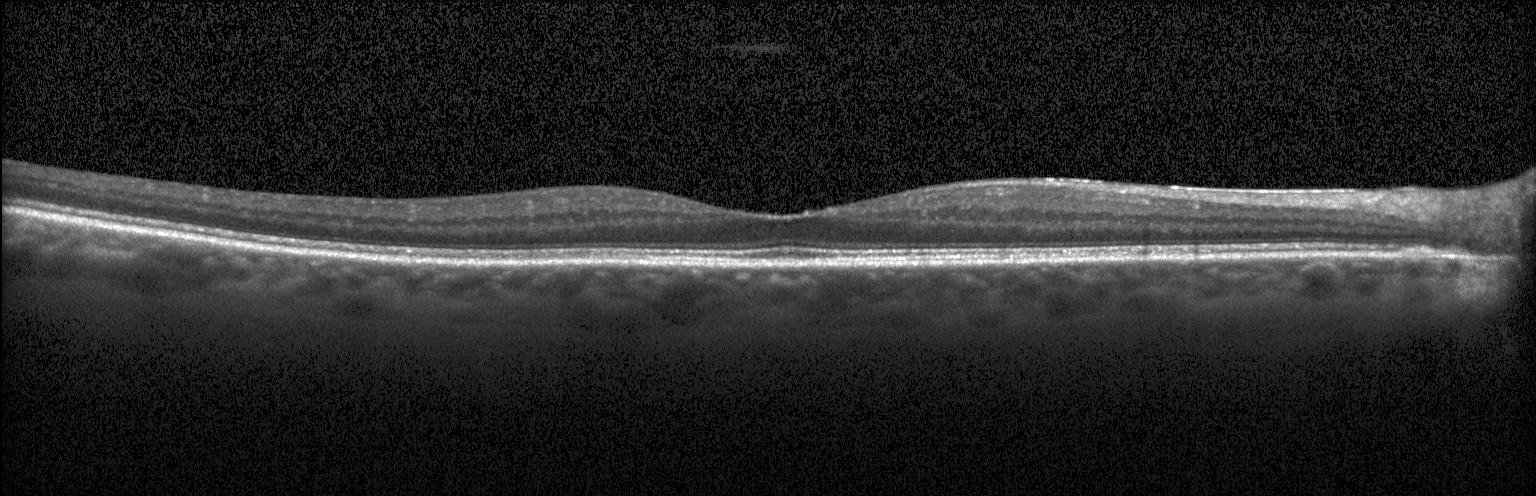
Spectral-domain OCT · OCT B-scan · instrument: Heidelberg Spectralis — Finding: no choroidal neovascularization, diabetic macular edema, or drusen.